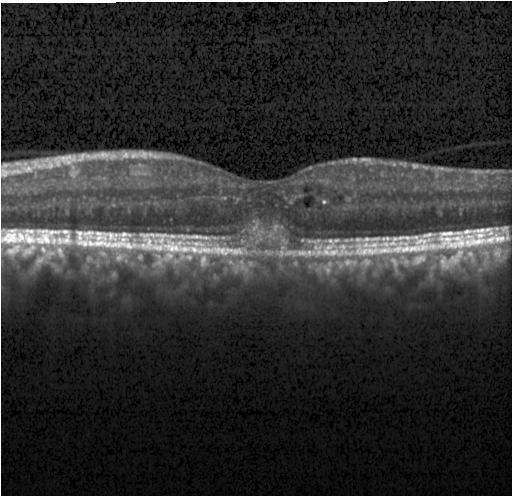 Optical coherence tomography B-scan.
Dx: choroidal neovascularization.